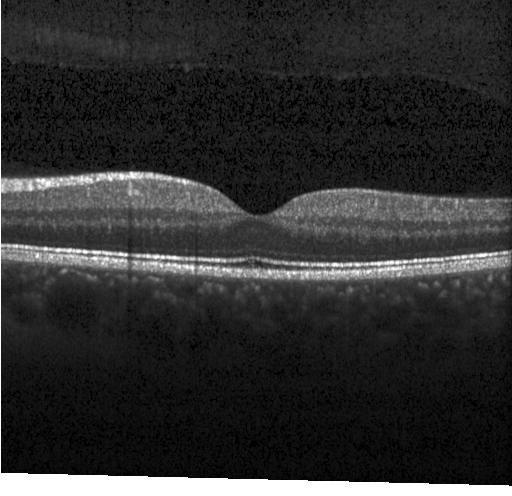
Macular OCT: no choroidal neovascularization, no diabetic macular edema, and no drusen.